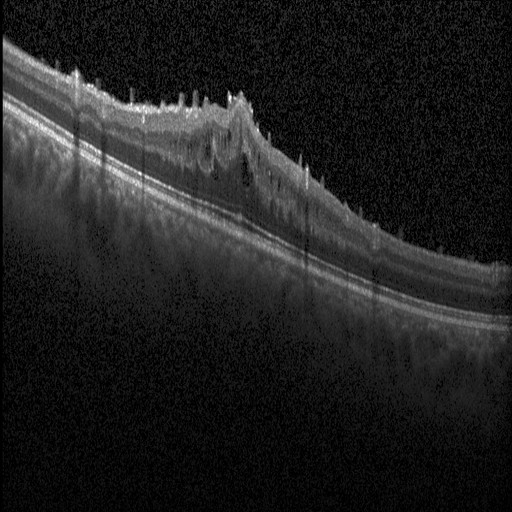

OCT B-scan — Finding: diabetic macular edema (DME).